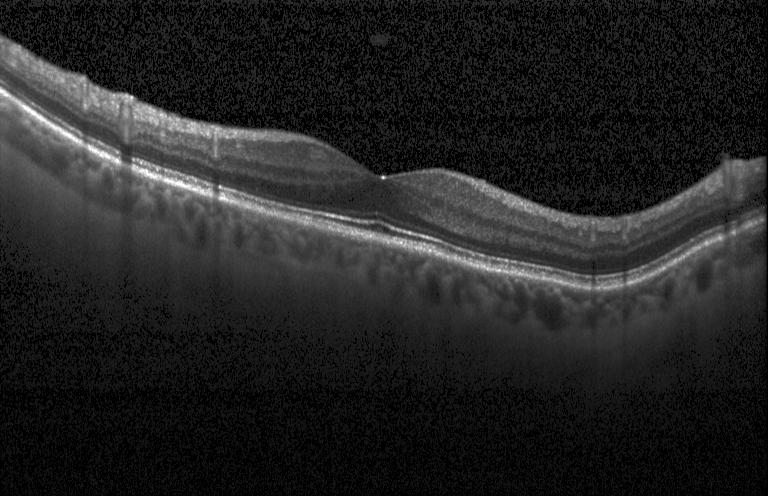 OCT B-scan · horizontal scan through the fovea
Diagnosis: neither choroidal neovascularization, diabetic macular edema, nor drusen.